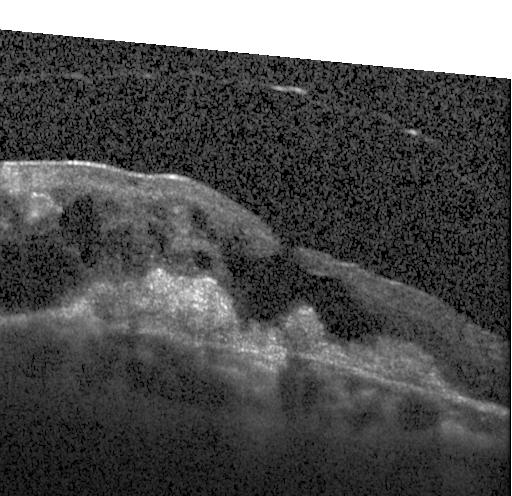 Optical coherence tomography scan. Diagnosis: a choroidal neovascular membrane.